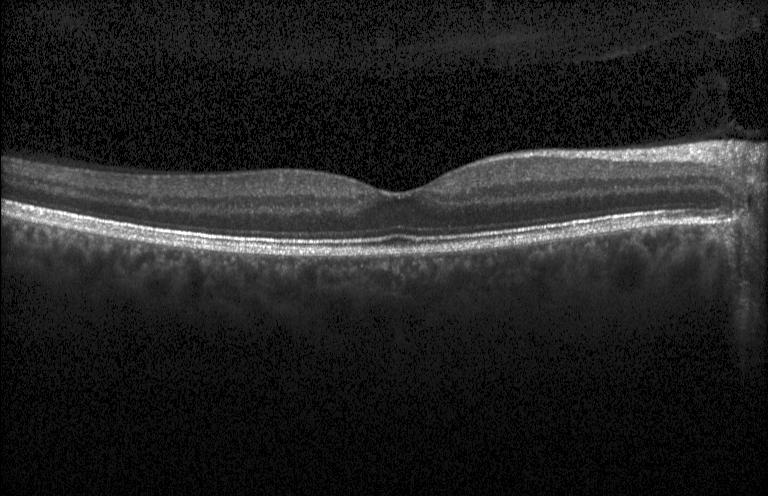
Centered on the fovea · retinal OCT cross-section · acquired on a Heidelberg Spectralis. Diagnosis: no choroidal neovascularization, diabetic macular edema, or drusen.